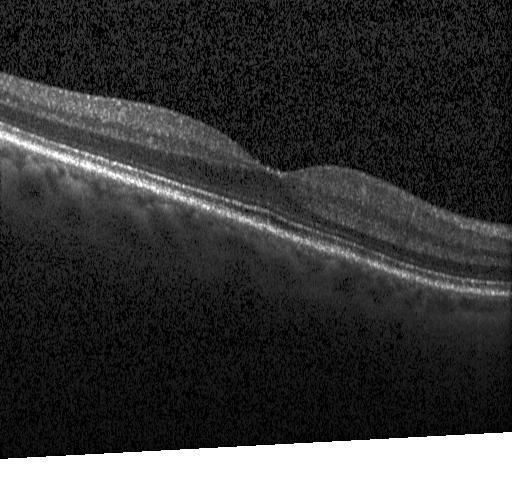
Diagnosis: no evidence of CNV, DME, or drusen.